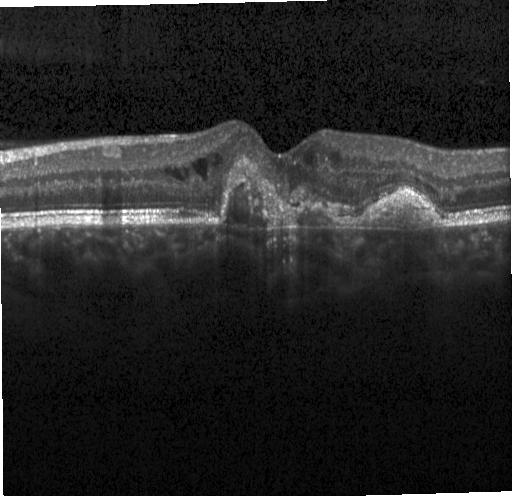

Centered on the fovea. Retinal OCT B-scan.
Diagnosis: a choroidal neovascular membrane.